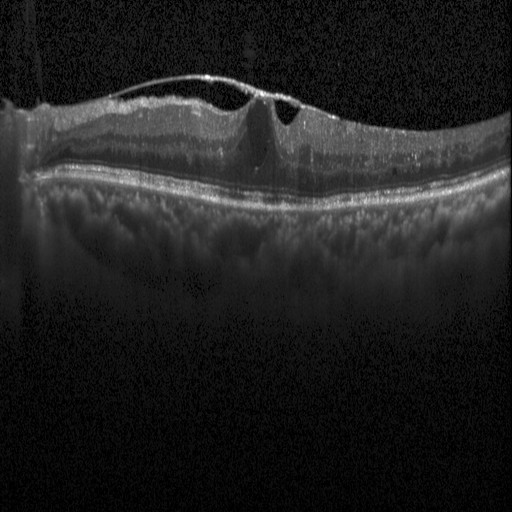 Retinal OCT cross-section showing diabetic macular edema.